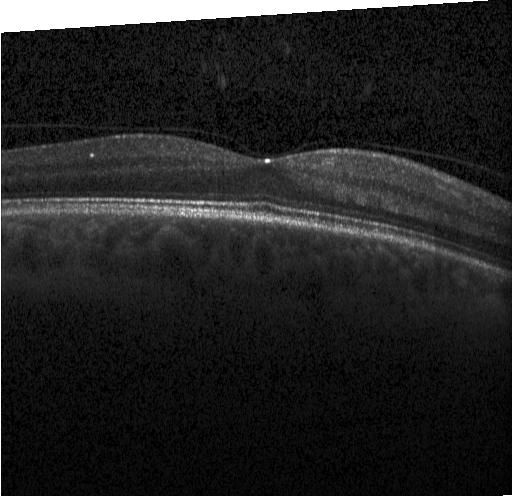

Fovea-centered; retinal OCT cross-section
Assessment: neither choroidal neovascularization, diabetic macular edema, nor drusen.